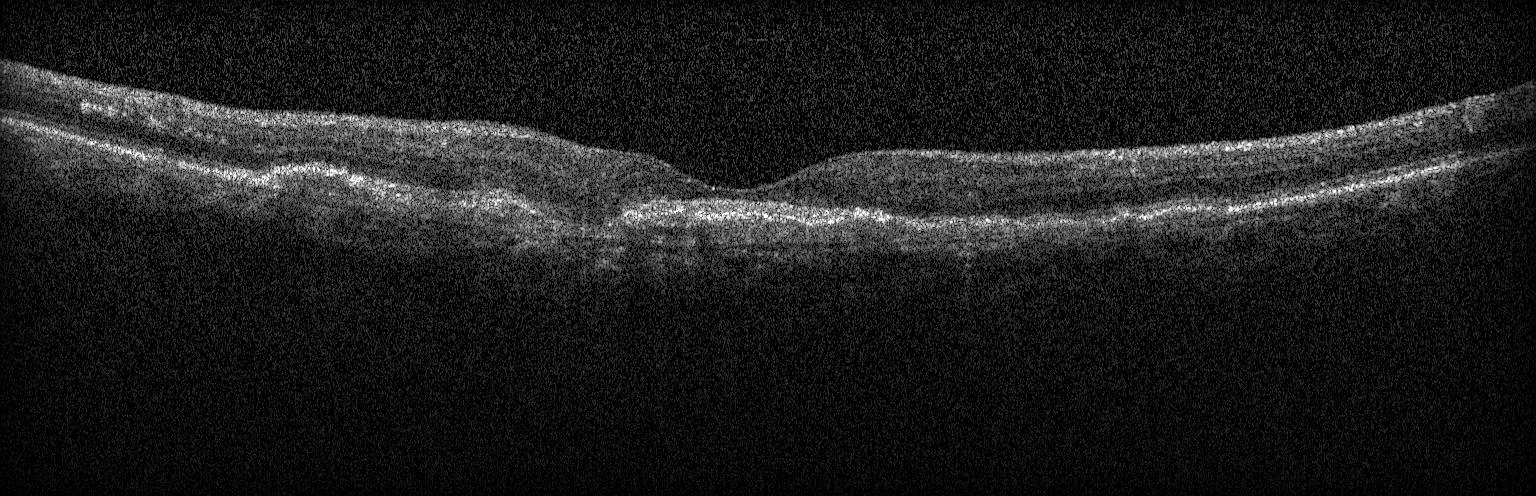 OCT B-scan. Assessment: choroidal neovascularization.